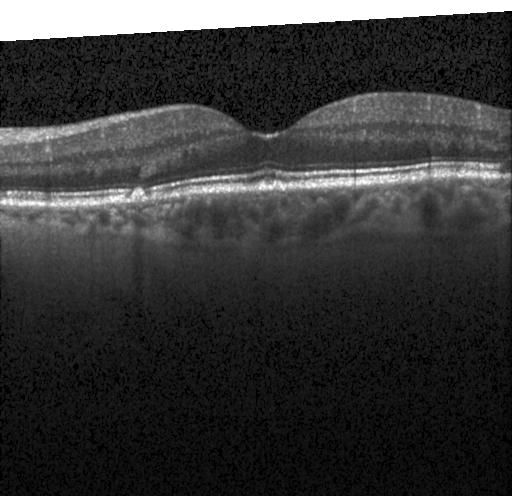

Diagnosis: multiple drusen.